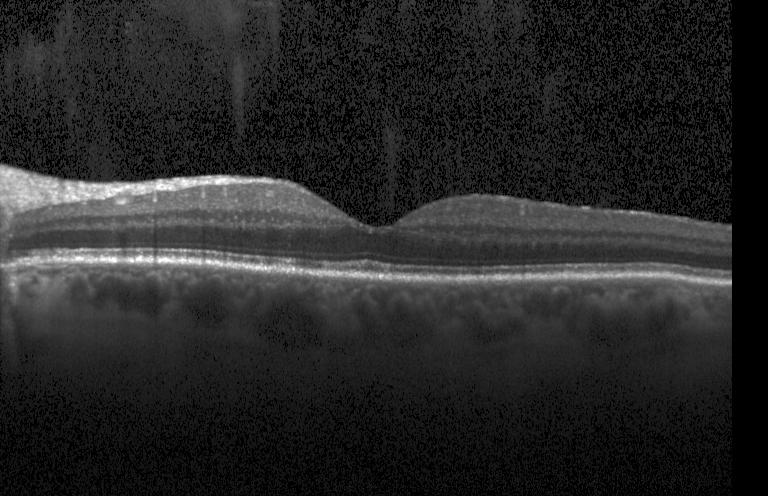
Macular OCT: neither choroidal neovascularization, diabetic macular edema, nor drusen.